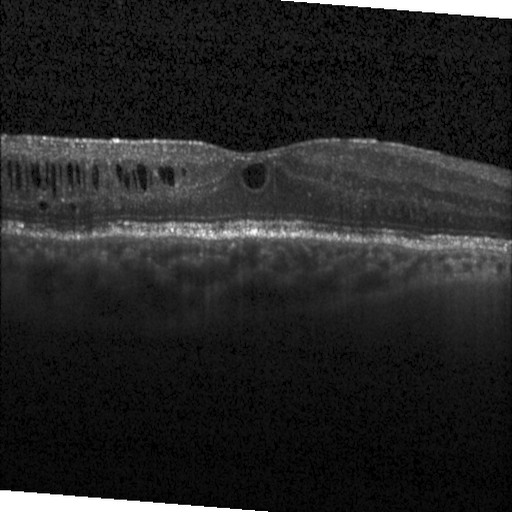
Retinal OCT B-scan.
Impression: diabetic macular edema.